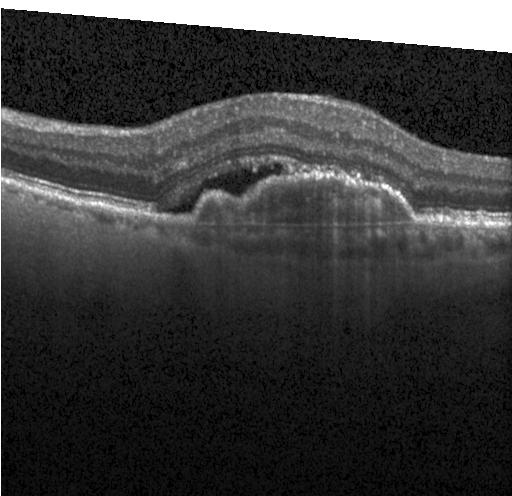

Fovea-centered; spectral-domain optical coherence tomography; optical coherence tomography scan; instrument: Heidelberg Spectralis. Assessment: choroidal neovascularization (CNV).